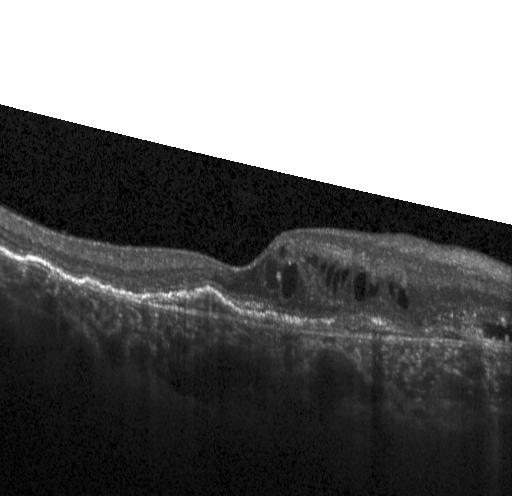 OCT finding: a choroidal neovascular membrane.